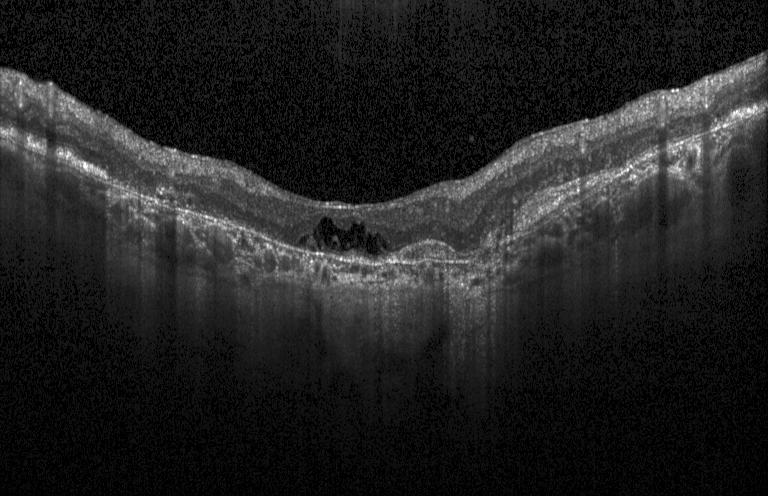
OCT B-scan. SD-OCT
Finding: choroidal neovascularization.